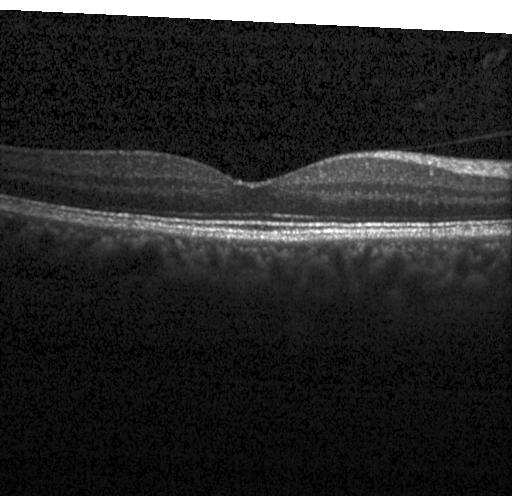
Macular OCT: no choroidal neovascularization, no diabetic macular edema, and no drusen.